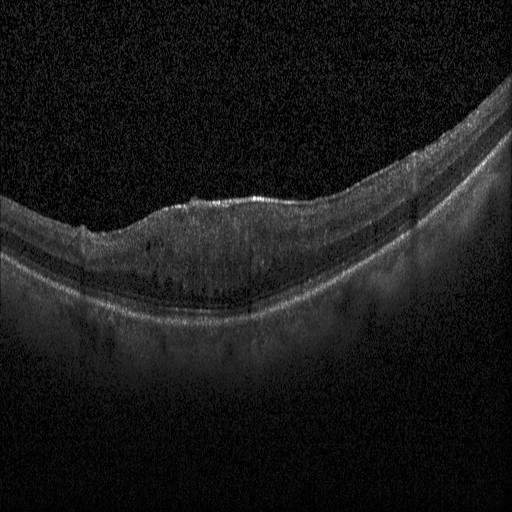 Heidelberg Spectralis; retinal OCT cross-section. Dx: DME.